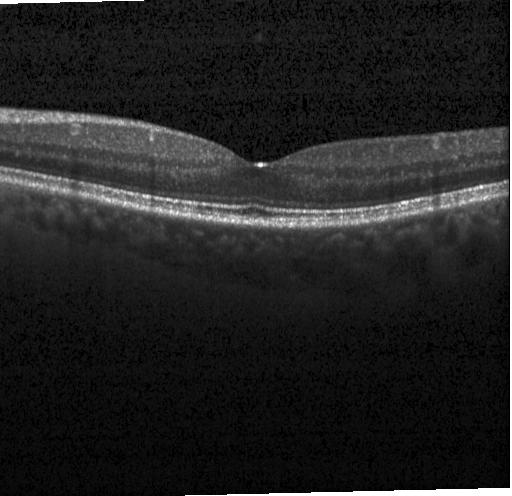

This B-scan demonstrates no CNV, DME, or drusen.